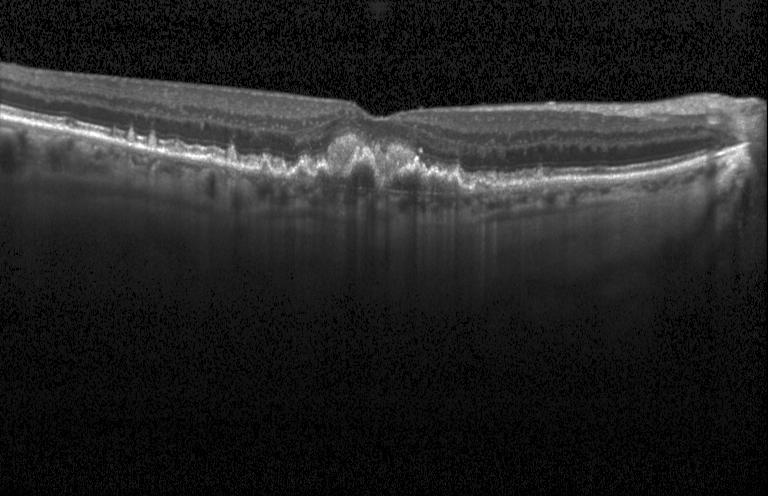

Finding: a choroidal neovascular membrane.